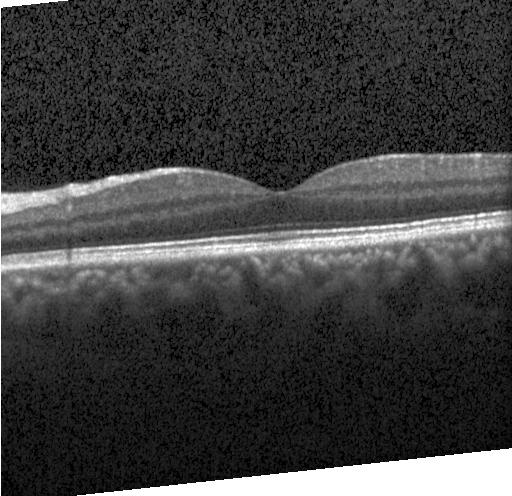 Macular scan; optical coherence tomography scan; Heidelberg Spectralis — OCT finding: neither CNV, DME, nor drusen.